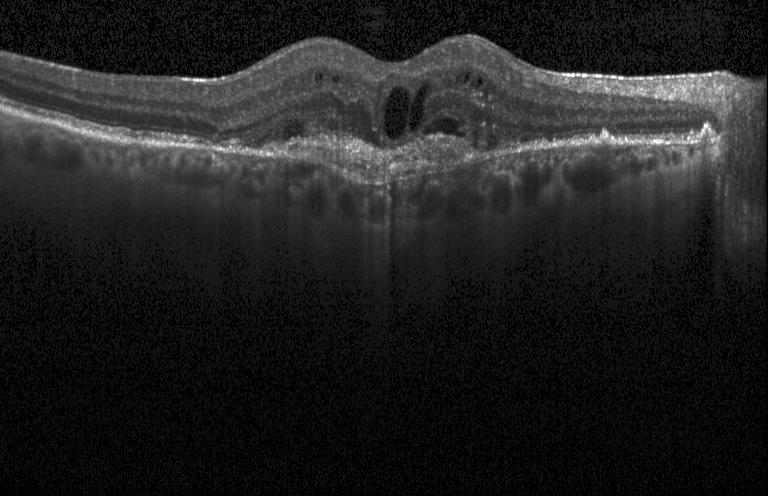
OCT B-scan, spectral-domain optical coherence tomography, Heidelberg Spectralis OCT system, macular scan.
This B-scan demonstrates choroidal neovascularization (CNV).